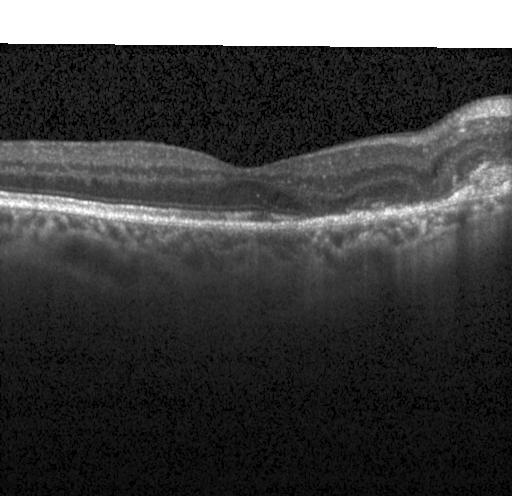

Finding: choroidal neovascularization.